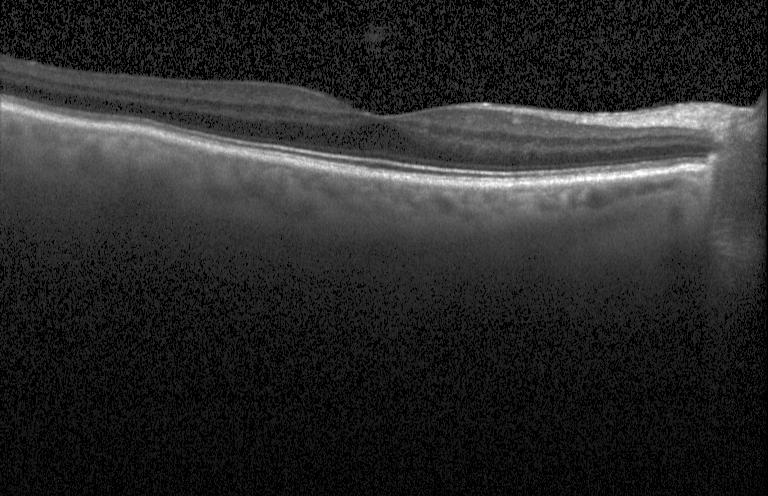

Macular OCT: no evidence of CNV, DME, or drusen.